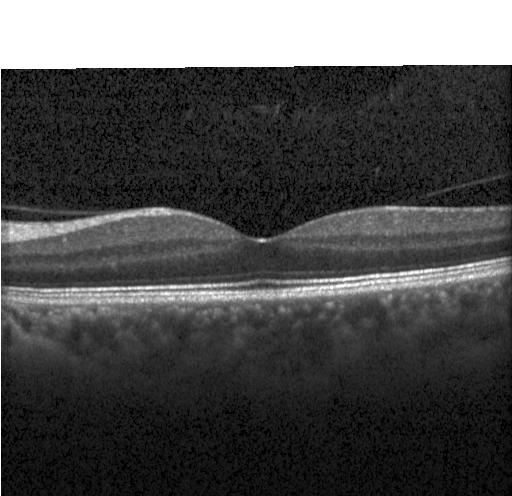 Optical coherence tomography B-scan · through the macula · SD-OCT · instrument: Heidelberg Spectralis — Finding: no choroidal neovascularization, no diabetic macular edema, and no drusen.